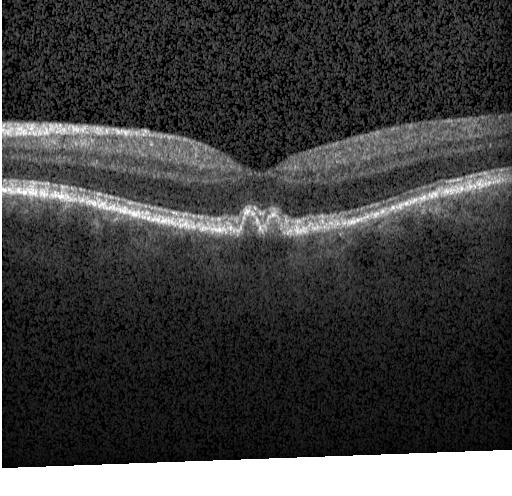
The scan shows drusen.